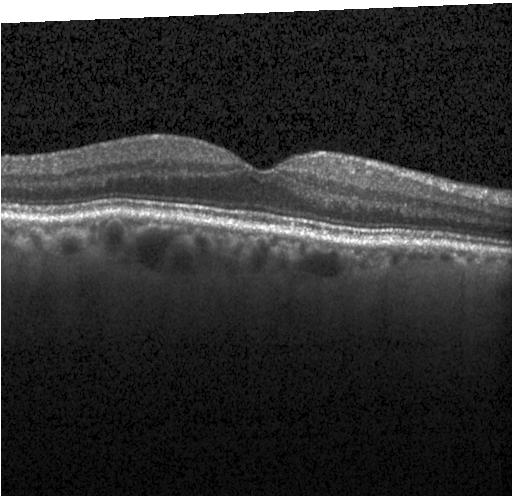
Retinal OCT cross-section. Heidelberg Spectralis — Impression: no CNV, no DME, and no drusen.